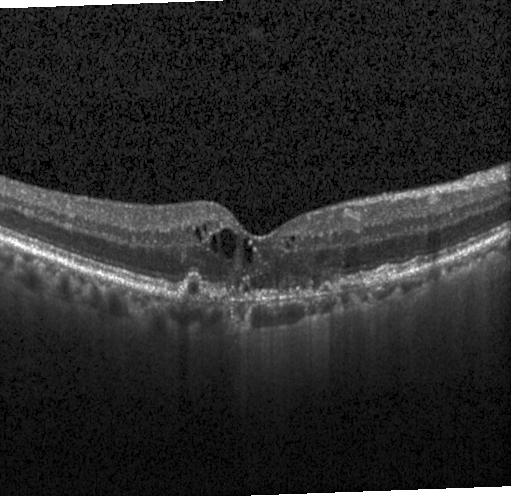

OCT scan showing choroidal neovascularization.